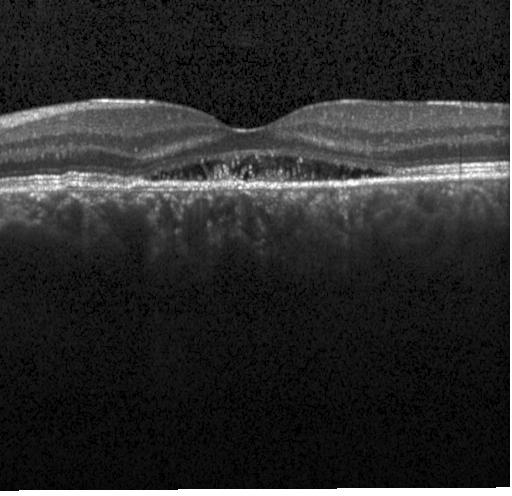

OCT scan showing CNV.